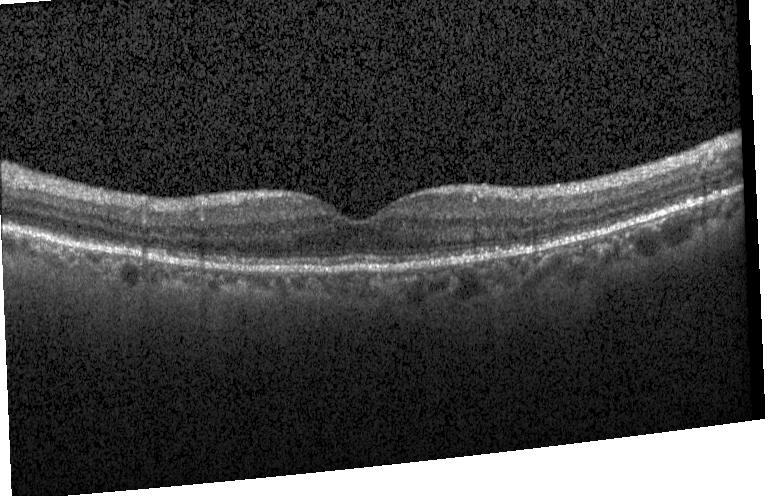

Impression: neither choroidal neovascularization, diabetic macular edema, nor drusen.